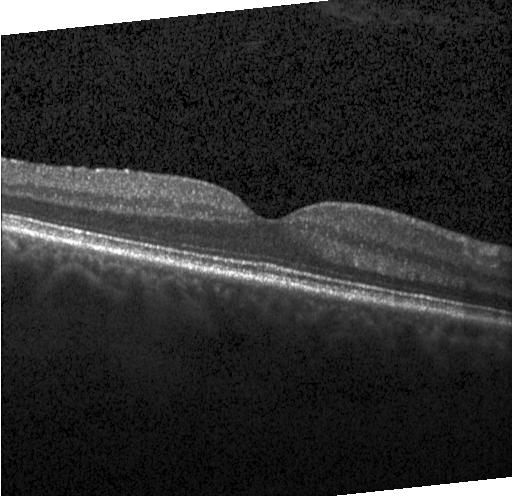 Heidelberg Spectralis. Spectral-domain optical coherence tomography. Macular scan. OCT line scan — OCT finding: no evidence of CNV, DME, or drusen.